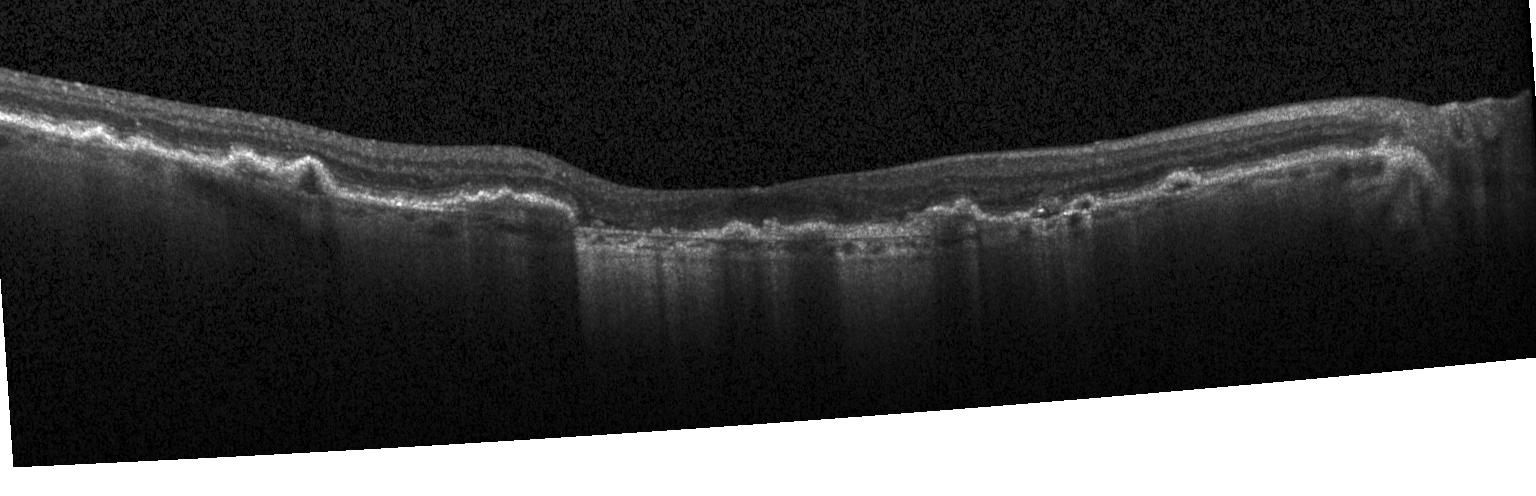
The scan shows a choroidal neovascular membrane.